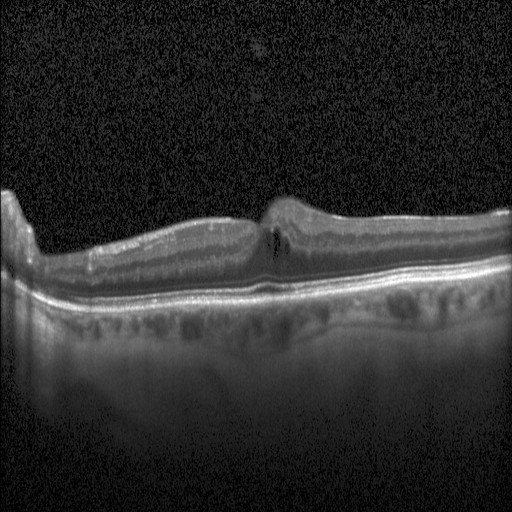 Dx: diabetic macular edema.